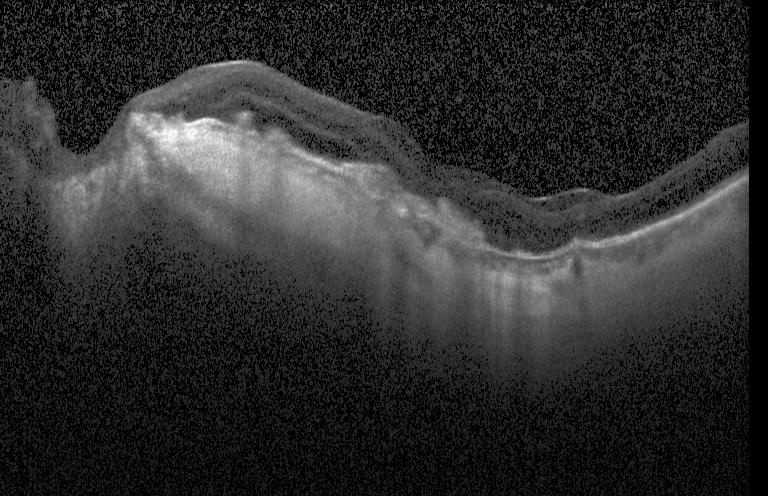
Retinal OCT cross-section. Instrument: Heidelberg Spectralis. Spectral-domain OCT
This B-scan demonstrates a choroidal neovascular membrane.